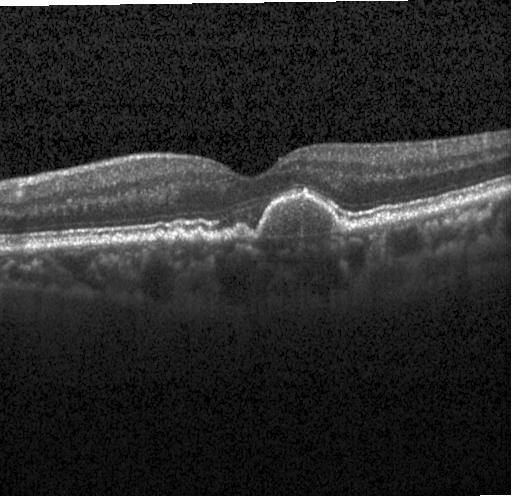 OCT line scan · SD-OCT · Heidelberg Spectralis · macular scan.
Finding: drusen.